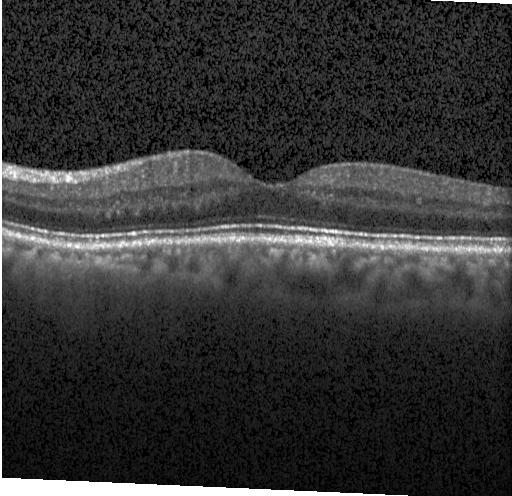 Instrument: Heidelberg Spectralis · optical coherence tomography B-scan · horizontal scan through the fovea
Impression: no evidence of choroidal neovascularization, diabetic macular edema, or drusen.